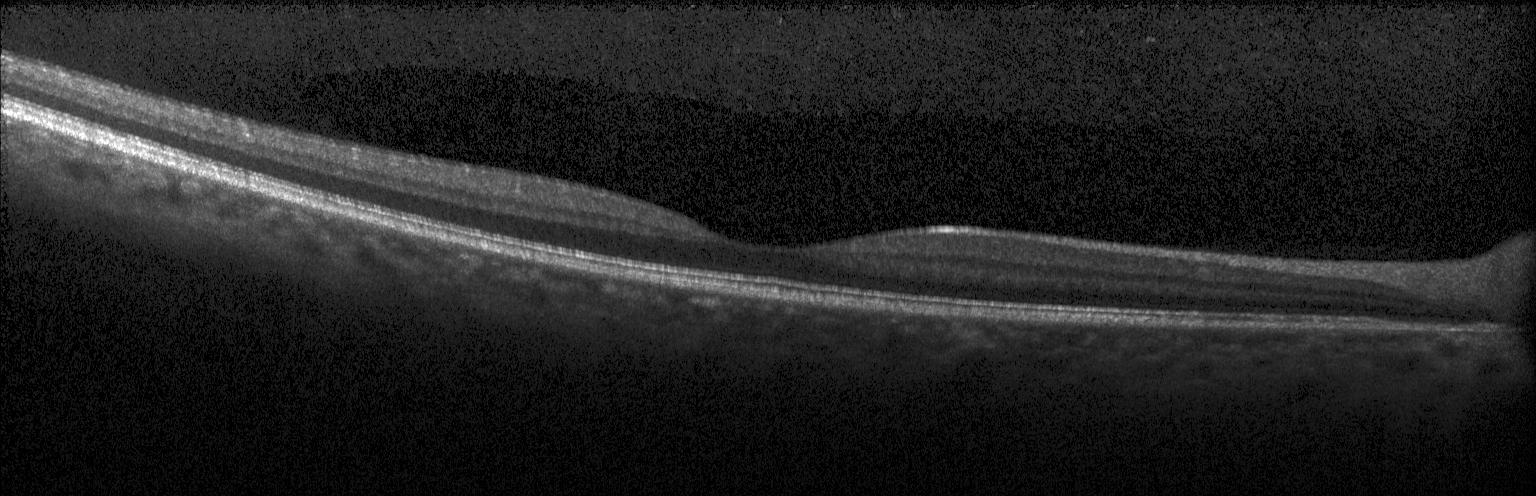

Retinal OCT B-scan; centered on the fovea; spectral-domain OCT — Assessment: no CNV, no DME, and no drusen.